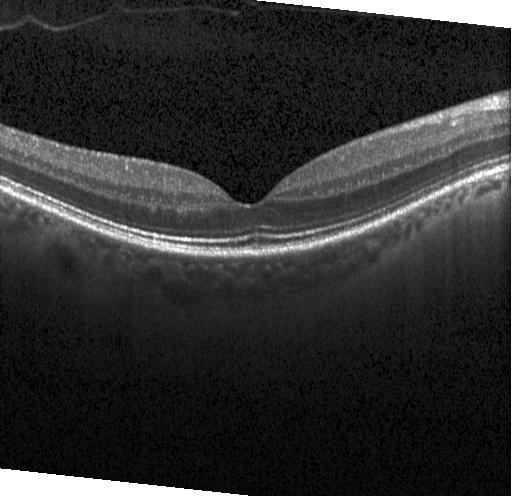 Macular OCT: no choroidal neovascularization, diabetic macular edema, or drusen.